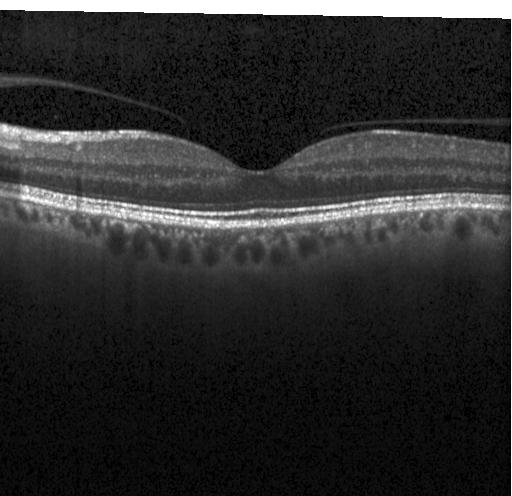 Optical coherence tomography scan; fovea-centered; SD-OCT.
No evidence of choroidal neovascularization, diabetic macular edema, or drusen.